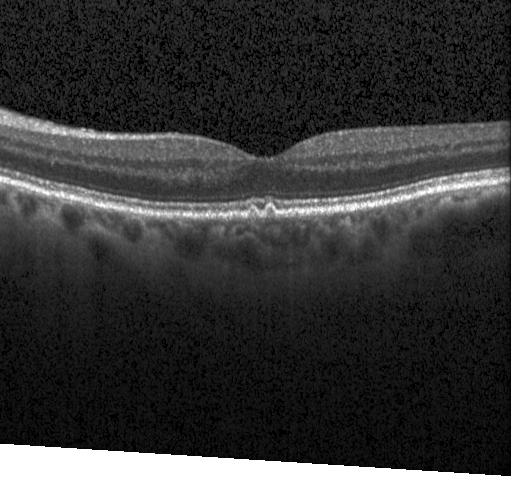 Impression: sub-RPE drusenoid deposits.